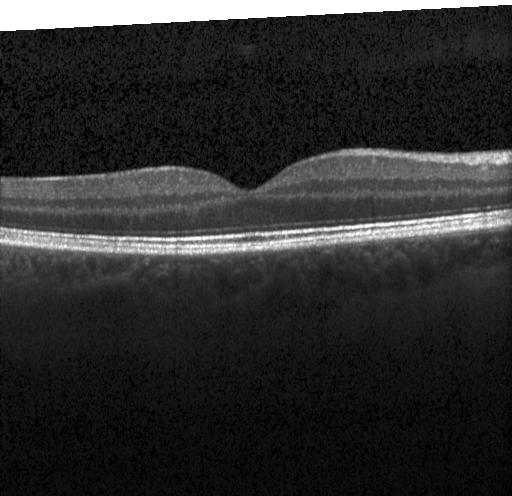 Optical coherence tomography scan; horizontal scan through the fovea; spectral-domain optical coherence tomography.
Finding: neither CNV, DME, nor drusen.